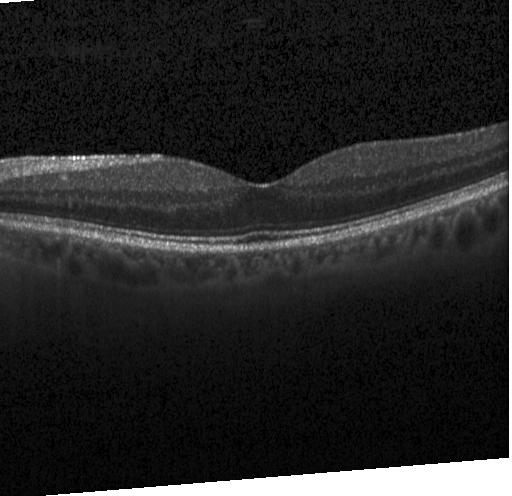 Retinal OCT B-scan.
This B-scan demonstrates no evidence of CNV, DME, or drusen.